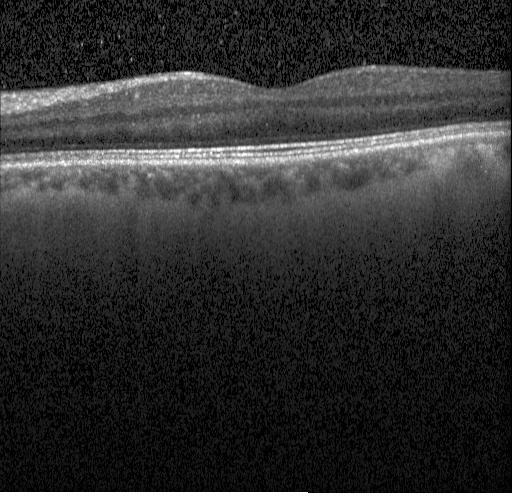 OCT B-scan. Diagnosis: no evidence of CNV, DME, or drusen.